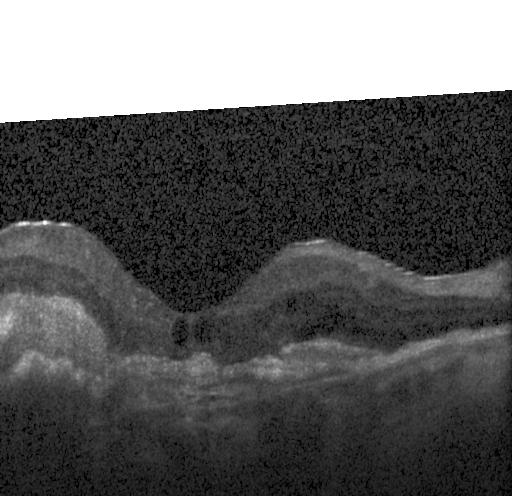 OCT scan showing a choroidal neovascular membrane.